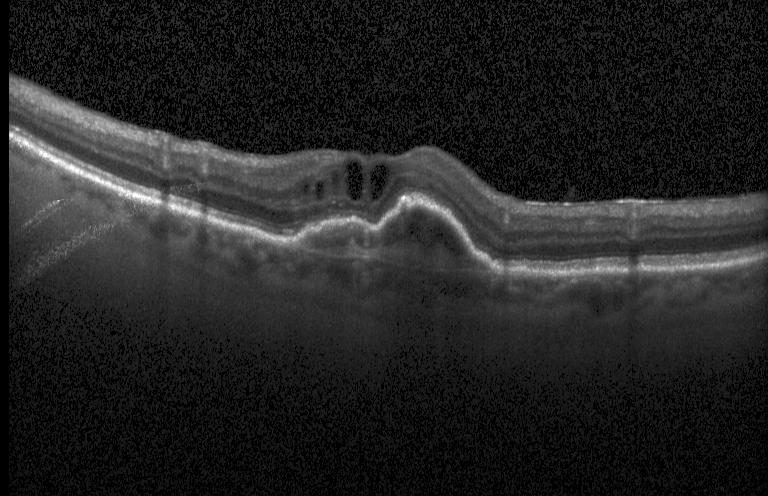 Centered on the fovea · retinal OCT cross-section.
Assessment: choroidal neovascularization.